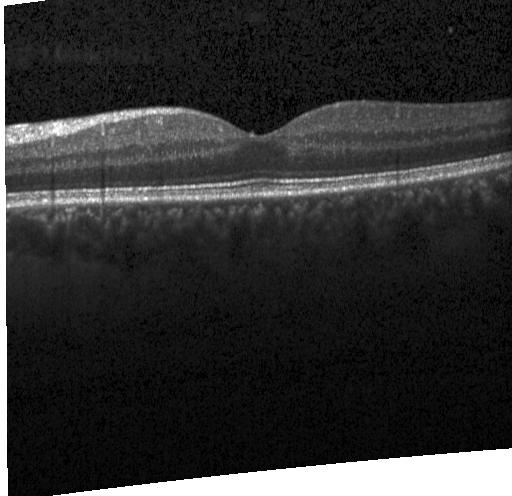
Diagnosis: no choroidal neovascularization, no diabetic macular edema, and no drusen.